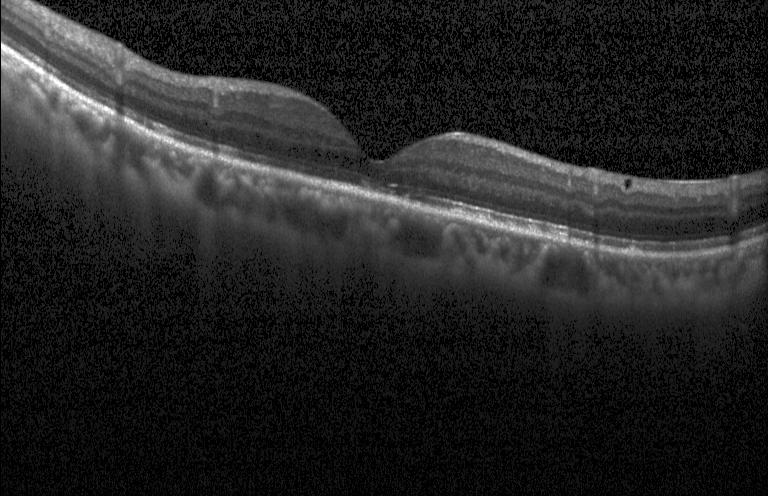

Spectral-domain OCT B-scan: no evidence of choroidal neovascularization, diabetic macular edema, or drusen.